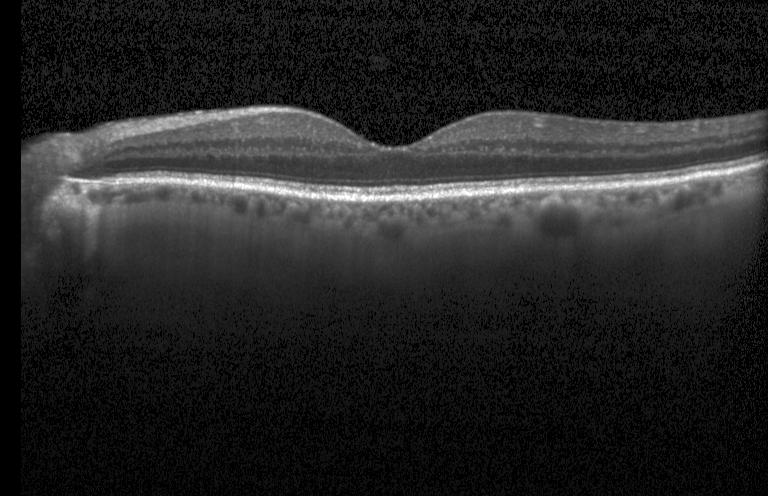 Acquired on a Heidelberg Spectralis · retinal OCT B-scan. Finding: no evidence of choroidal neovascularization, diabetic macular edema, or drusen.